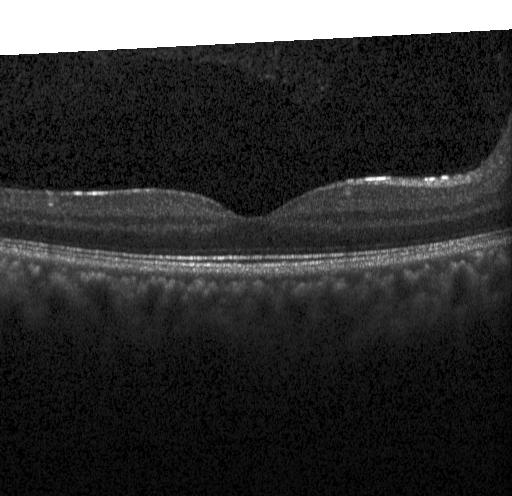 Heidelberg Spectralis · retinal OCT B-scan · centered on the fovea · SD-OCT
Finding: no CNV, no DME, and no drusen.